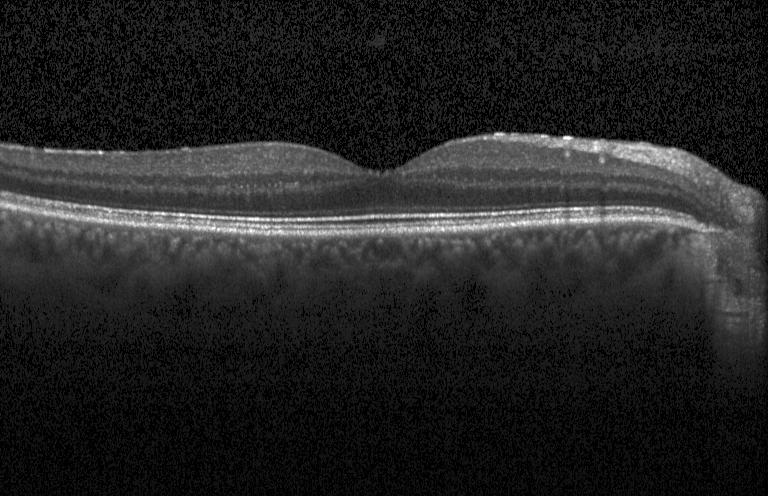
Spectral-domain OCT · Heidelberg Spectralis · OCT line scan — Finding: neither choroidal neovascularization, diabetic macular edema, nor drusen.